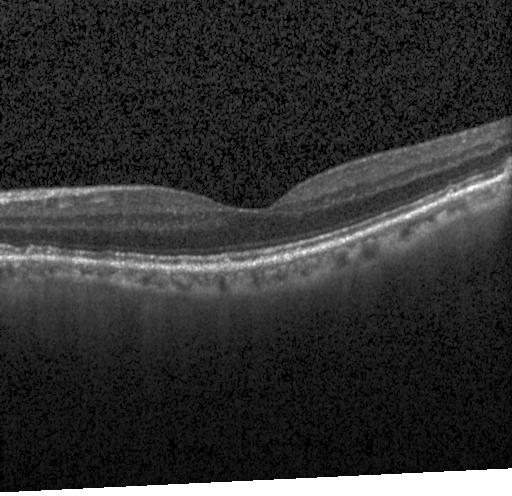

OCT B-scan; spectral-domain OCT; through the macula — This B-scan demonstrates no choroidal neovascularization, diabetic macular edema, or drusen.